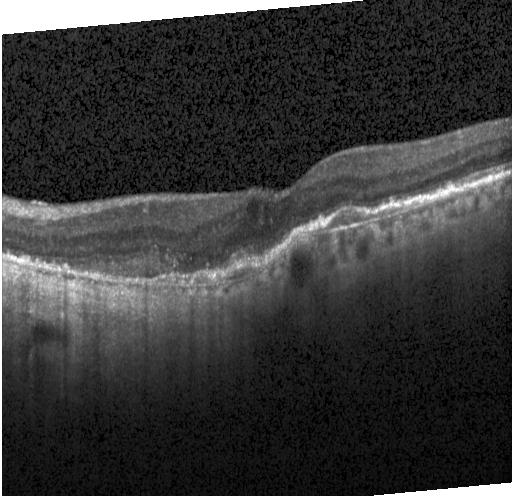 OCT B-scan. Spectral-domain optical coherence tomography. Heidelberg Spectralis. Macular scan.
Finding: a choroidal neovascular membrane.